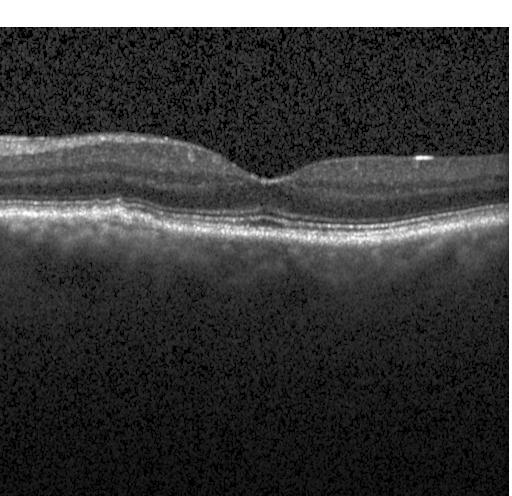 Dx: multiple drusen.